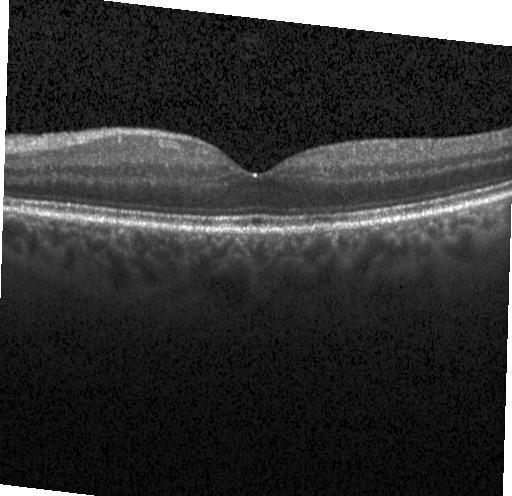

SD-OCT. Optical coherence tomography scan. Heidelberg Spectralis.
The scan shows no choroidal neovascularization, no diabetic macular edema, and no drusen.